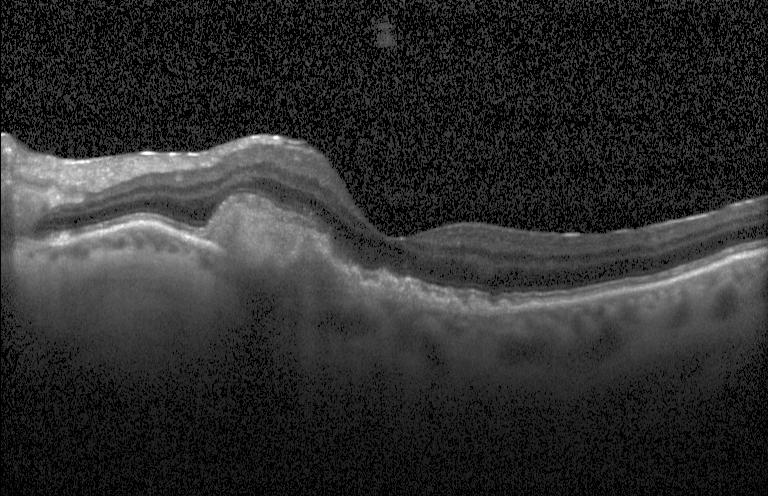 Optical coherence tomography B-scan · spectral-domain OCT · centered on the fovea
This B-scan demonstrates a choroidal neovascular membrane.